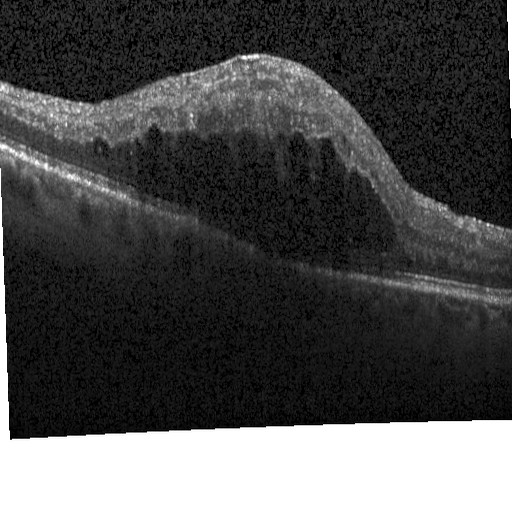
Macular OCT: DME.